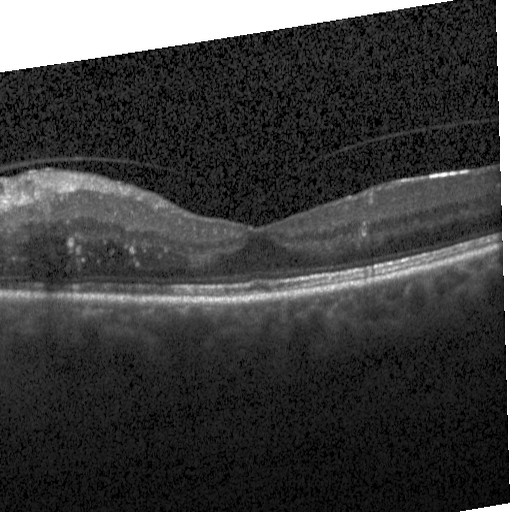

OCT finding: diabetic macular edema.